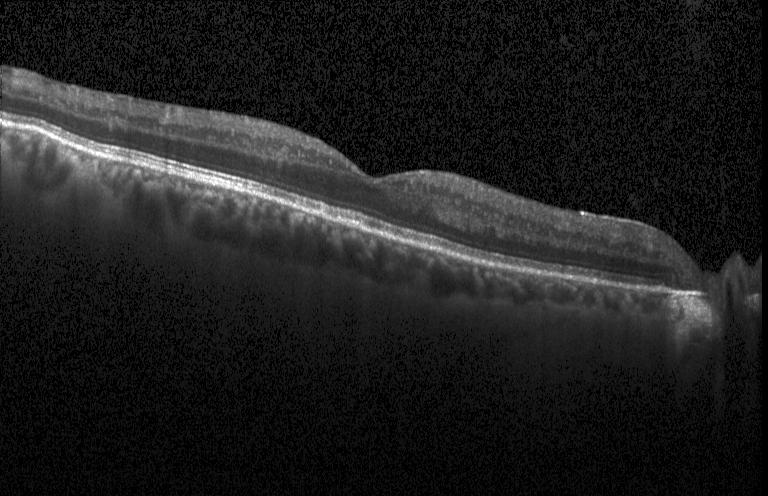

OCT line scan
OCT finding: no evidence of choroidal neovascularization, diabetic macular edema, or drusen.